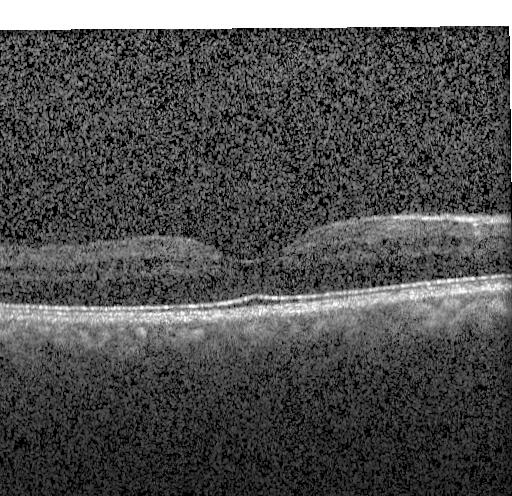
Optical coherence tomography scan — Impression: no evidence of CNV, DME, or drusen.